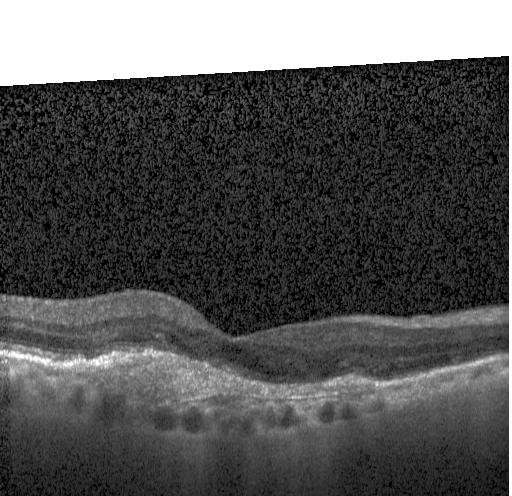 Spectral-domain OCT; instrument: Heidelberg Spectralis; macular scan; retinal OCT cross-section.
A choroidal neovascular membrane.